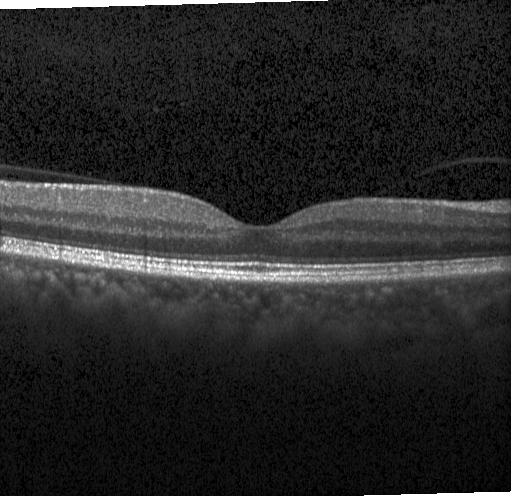

Impression: no choroidal neovascularization, no diabetic macular edema, and no drusen.